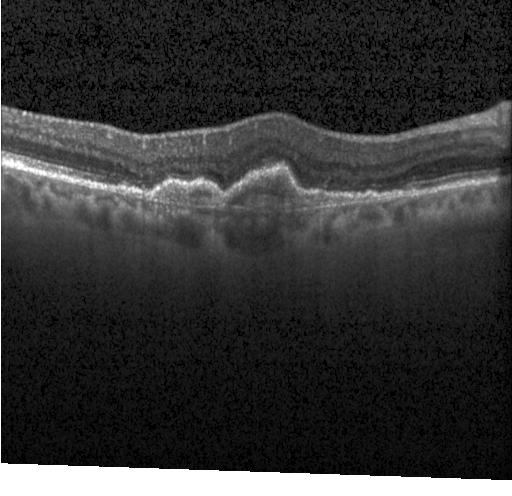

Centered on the fovea · retinal OCT cross-section
Assessment: a choroidal neovascular membrane.